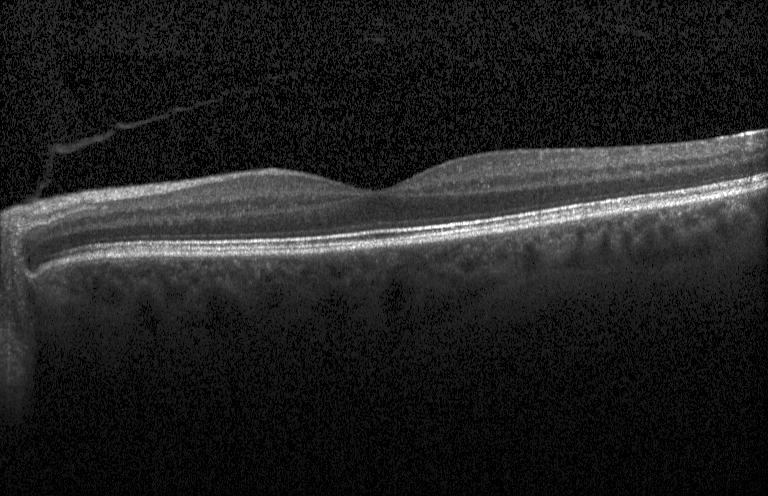
Heidelberg Spectralis OCT system. Spectral-domain optical coherence tomography. Horizontal scan through the fovea. OCT line scan — This B-scan demonstrates neither CNV, DME, nor drusen.